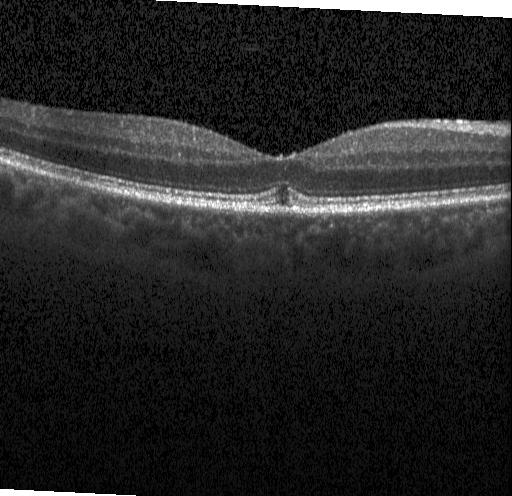 Retinal OCT B-scan, centered on the fovea — OCT finding: neither choroidal neovascularization, diabetic macular edema, nor drusen.